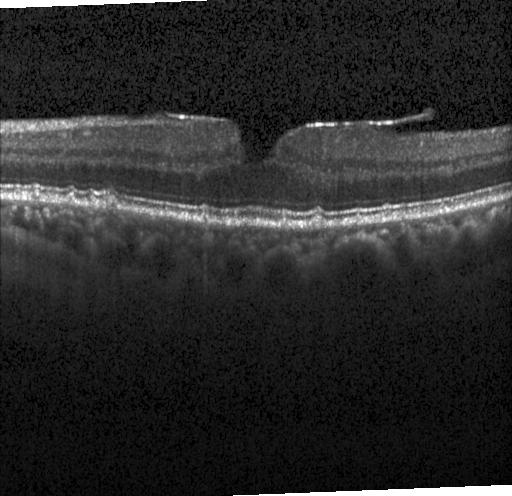
SD-OCT, optical coherence tomography B-scan — Impression: drusen.